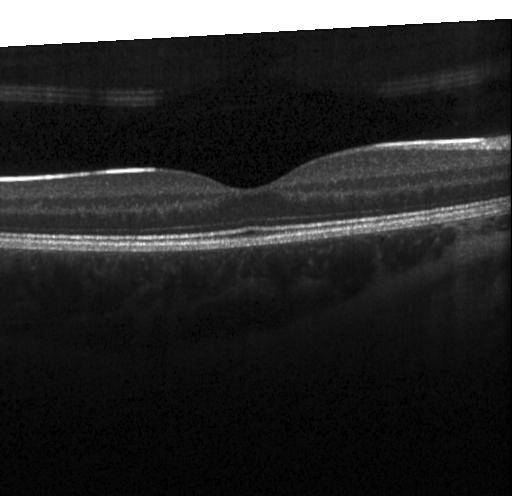
Macular scan, spectral-domain OCT, Heidelberg Spectralis OCT system, optical coherence tomography scan — OCT finding: no choroidal neovascularization, no diabetic macular edema, and no drusen.